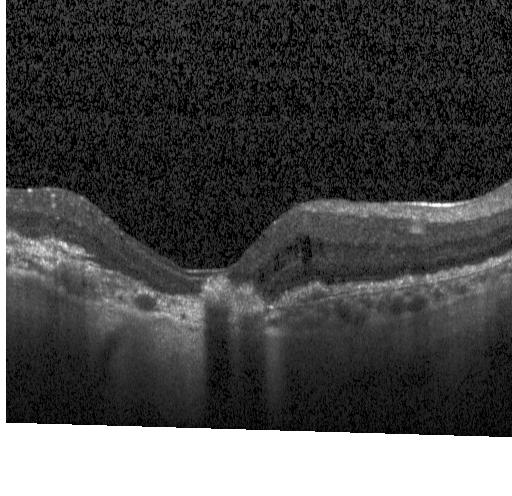 Retinal OCT cross-section showing CNV.